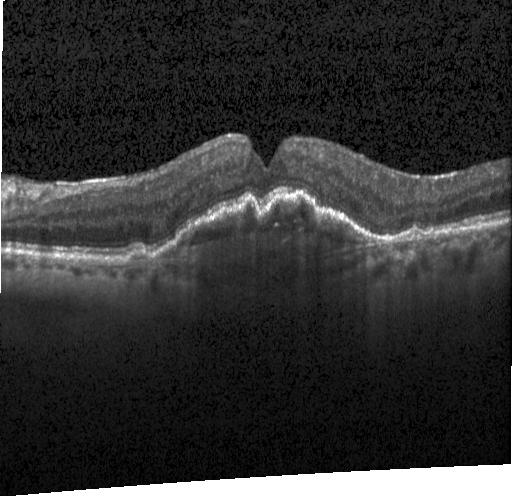
Optical coherence tomography B-scan · Heidelberg Spectralis OCT system · through the macula · spectral-domain OCT.
OCT finding: a choroidal neovascular membrane.